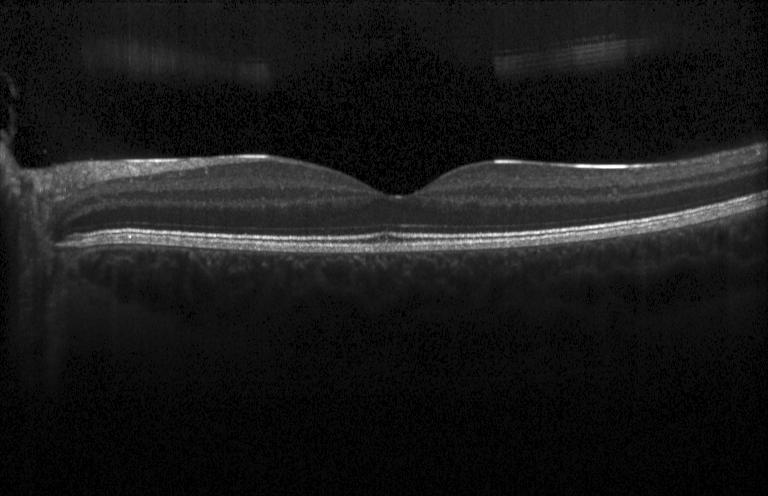 Fovea-centered, retinal OCT cross-section, spectral-domain optical coherence tomography — Neither choroidal neovascularization, diabetic macular edema, nor drusen.